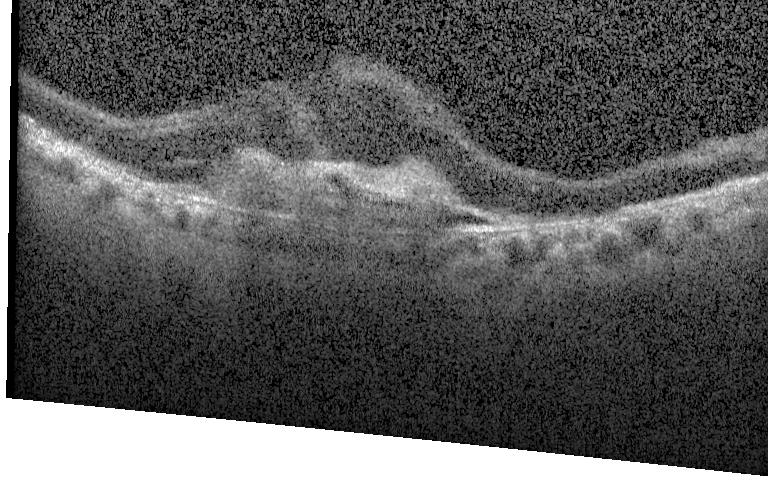

Through the macula. Optical coherence tomography scan. Acquired on a Heidelberg Spectralis. Macular OCT: choroidal neovascularization.